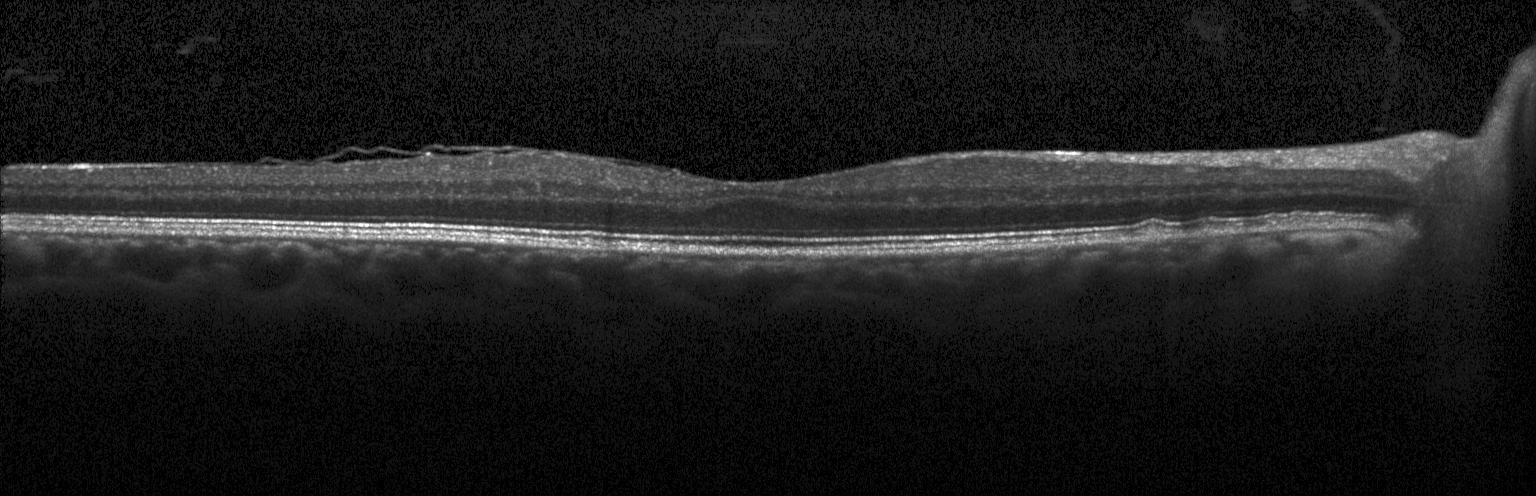
Retinal OCT cross-section showing sub-RPE drusenoid deposits.